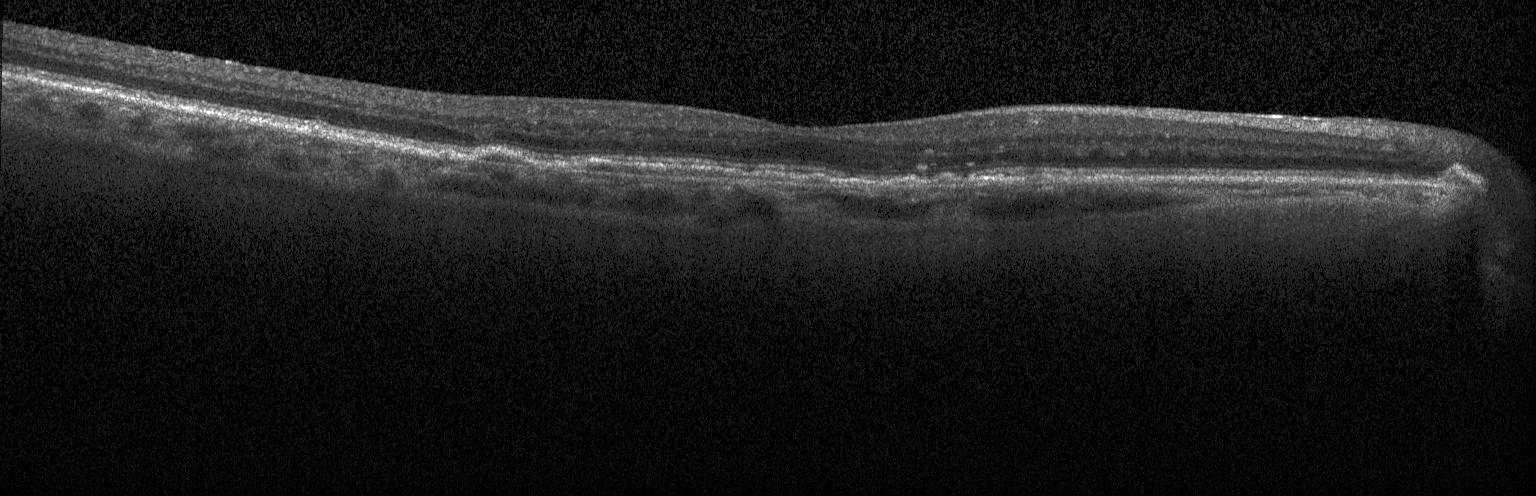 Dx: CNV.